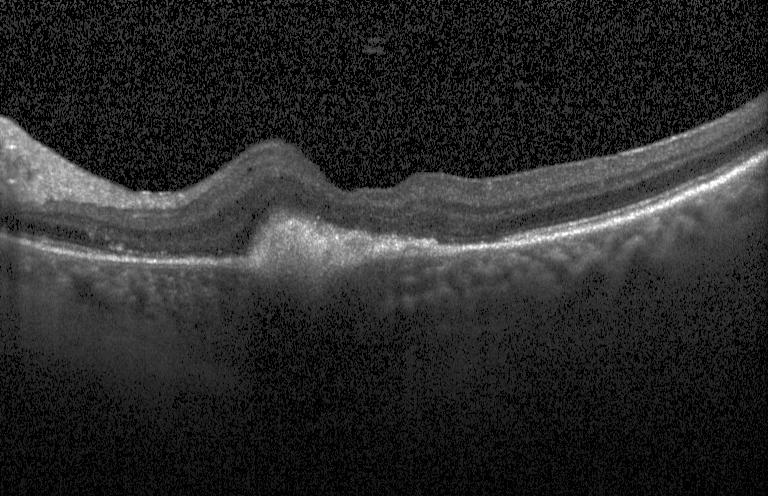 Heidelberg Spectralis OCT system · OCT B-scan · SD-OCT. Finding: choroidal neovascularization.